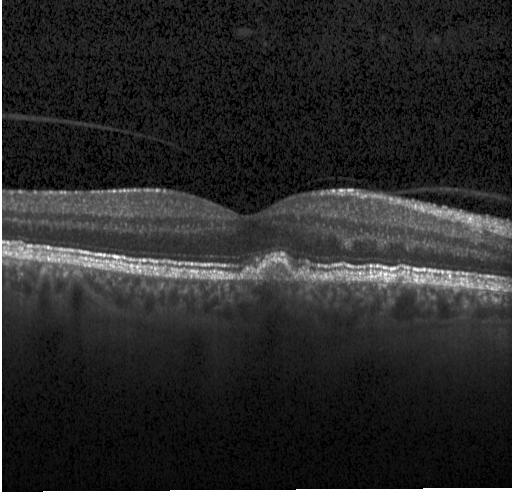

Impression: sub-RPE drusenoid deposits.